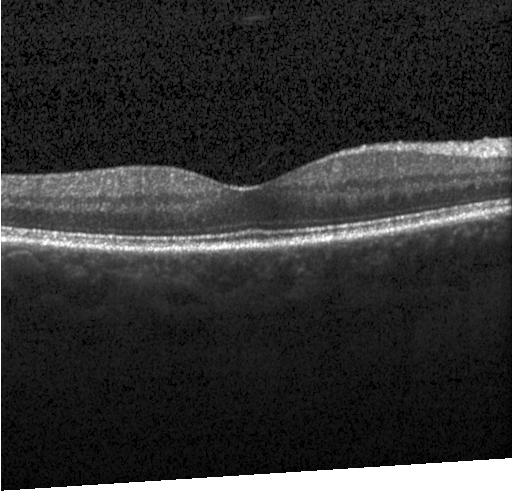
Impression: no CNV, no DME, and no drusen.